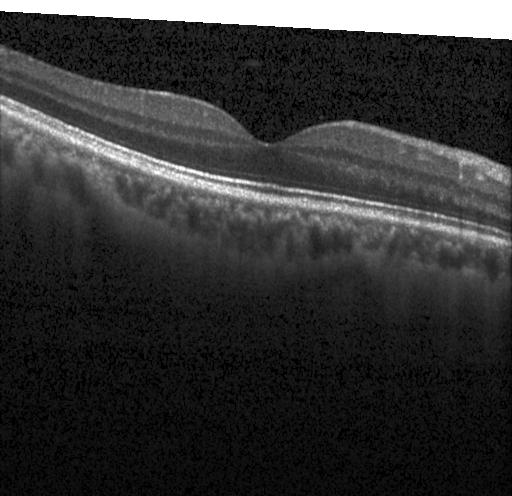
The scan shows neither choroidal neovascularization, diabetic macular edema, nor drusen.